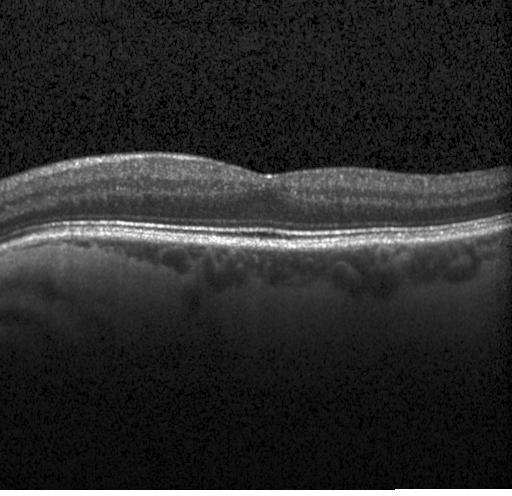 Finding: no evidence of CNV, DME, or drusen.